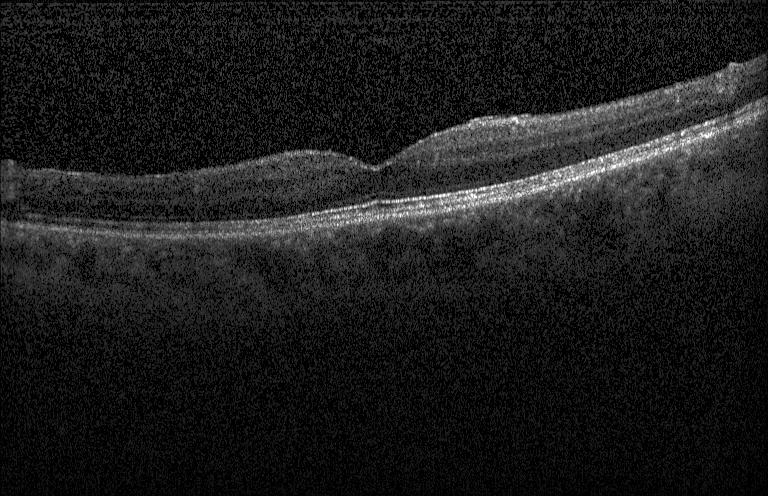 Retinal OCT cross-section, spectral-domain optical coherence tomography, instrument: Heidelberg Spectralis — OCT finding: no CNV, DME, or drusen.